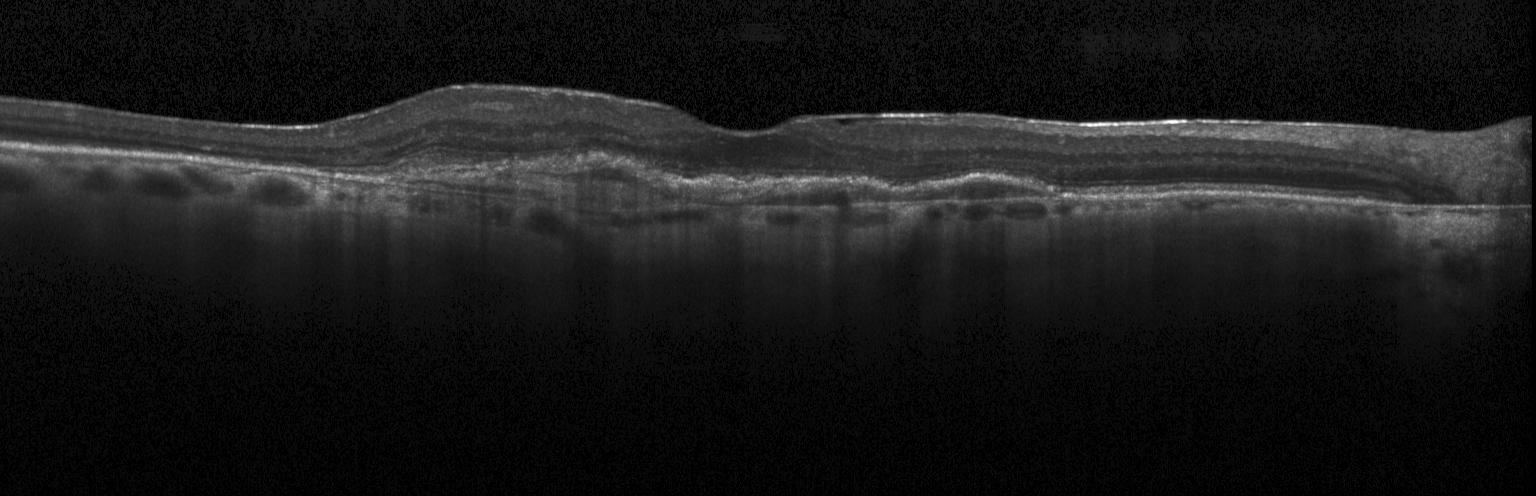

Retinal OCT cross-section, acquired on a Heidelberg Spectralis, spectral-domain OCT, horizontal scan through the fovea — Finding: a choroidal neovascular membrane.